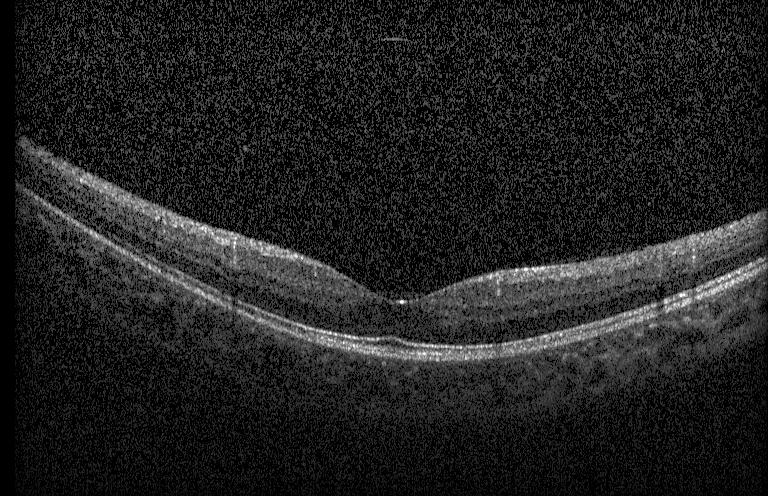 Retinal OCT cross-section showing neither CNV, DME, nor drusen.